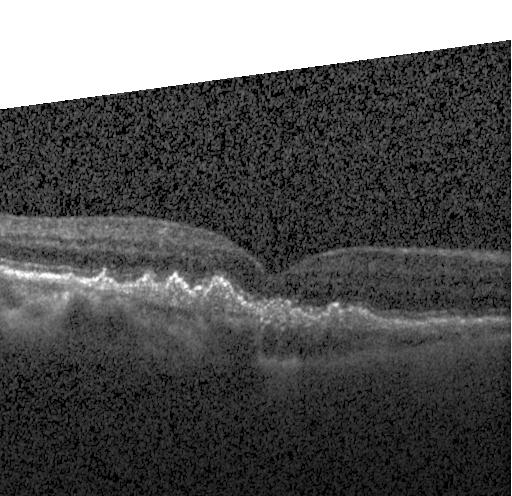 Diagnosis: choroidal neovascularization (CNV).